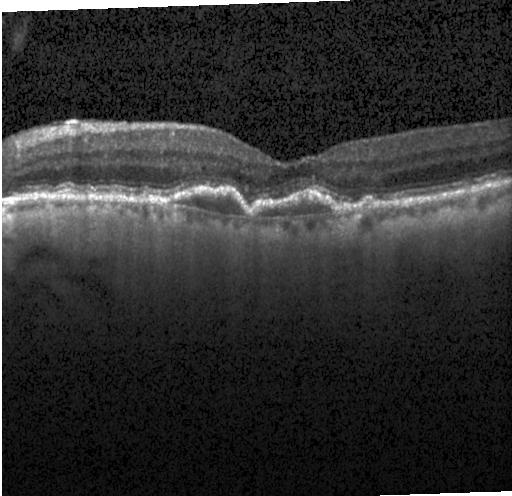
Acquired on a Heidelberg Spectralis · OCT B-scan · fovea-centered · SD-OCT
Dx: choroidal neovascularization (CNV).